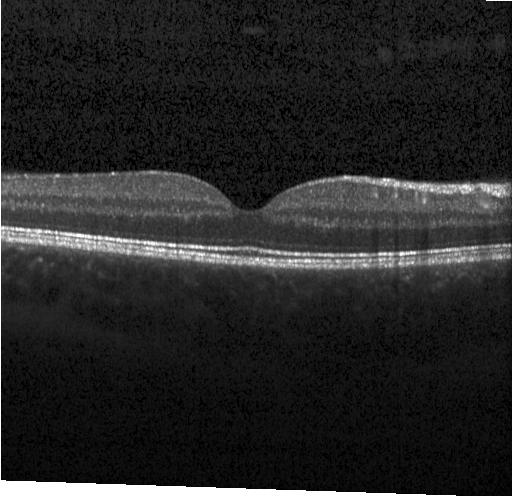
Optical coherence tomography B-scan — Dx: no choroidal neovascularization, diabetic macular edema, or drusen.